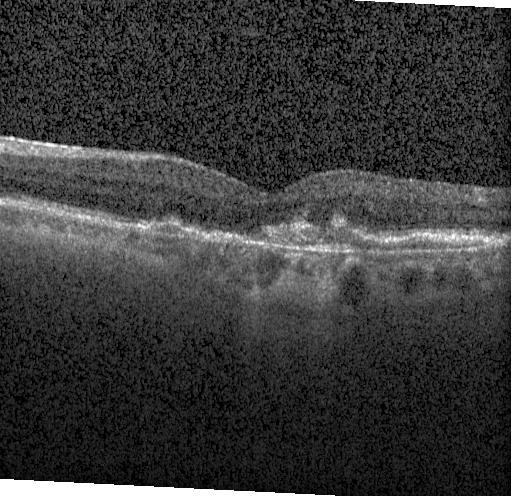
Finding: choroidal neovascularization.